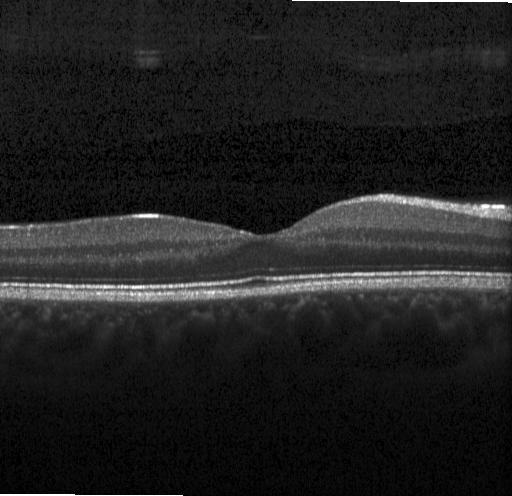
Impression: no CNV, DME, or drusen.